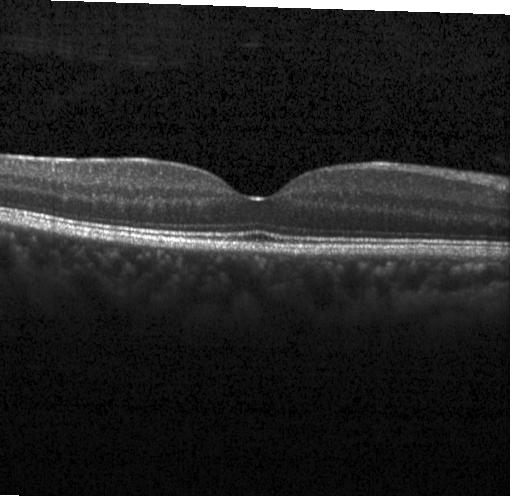

Optical coherence tomography scan
Finding: no CNV, DME, or drusen.